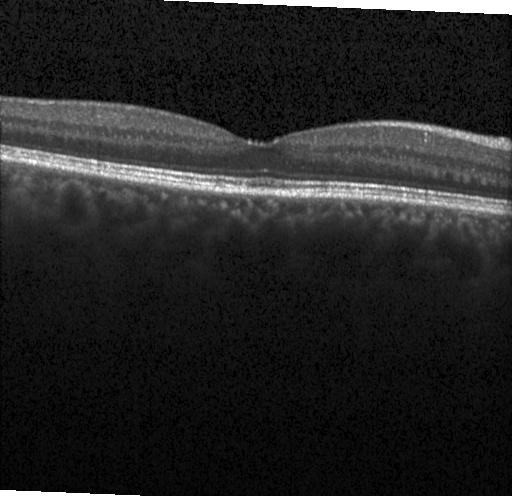
Heidelberg Spectralis OCT system · retinal OCT B-scan · macular scan.
The scan shows no evidence of choroidal neovascularization, diabetic macular edema, or drusen.